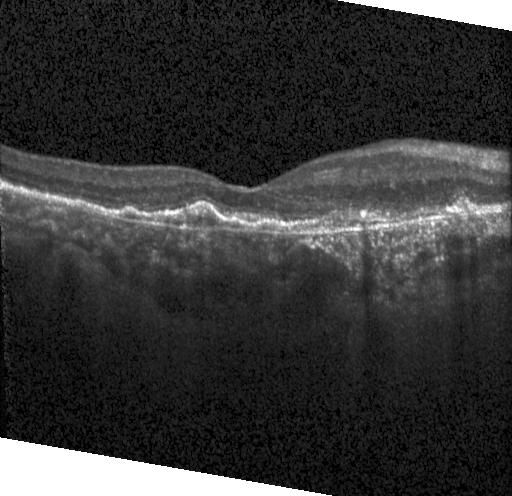
OCT B-scan — Finding: choroidal neovascularization.